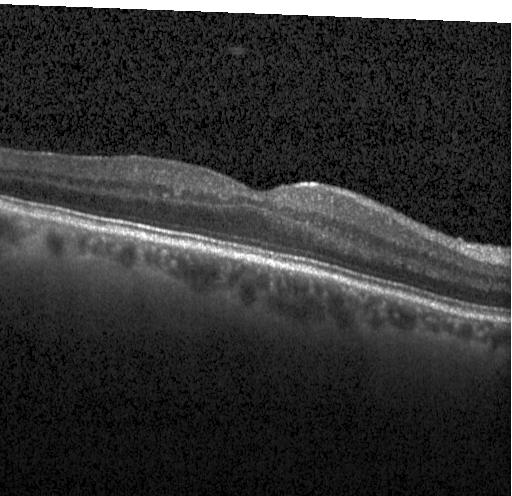 Instrument: Heidelberg Spectralis, retinal OCT cross-section. Impression: neither choroidal neovascularization, diabetic macular edema, nor drusen.